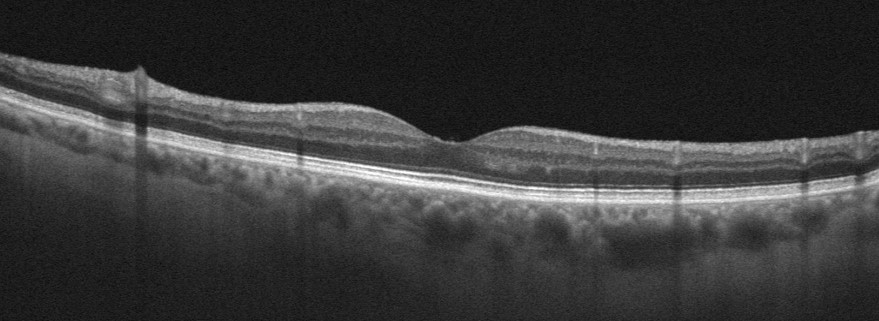 Instrument: Optovue Avanti RTVue XR, retinal OCT B-scan.
Diagnosis: no AMD, DME, ERM, RAO, RVO, or VID.